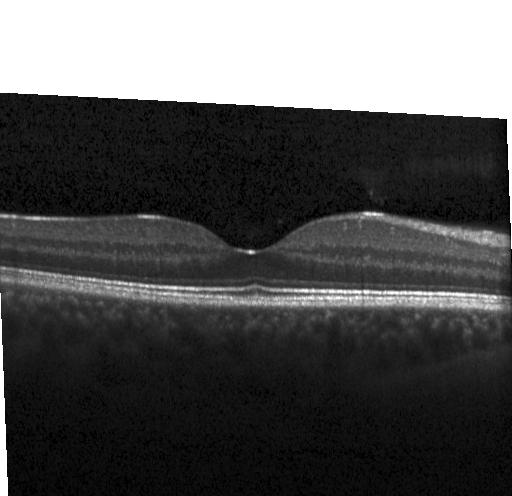

Retinal OCT B-scan
This B-scan demonstrates neither CNV, DME, nor drusen.